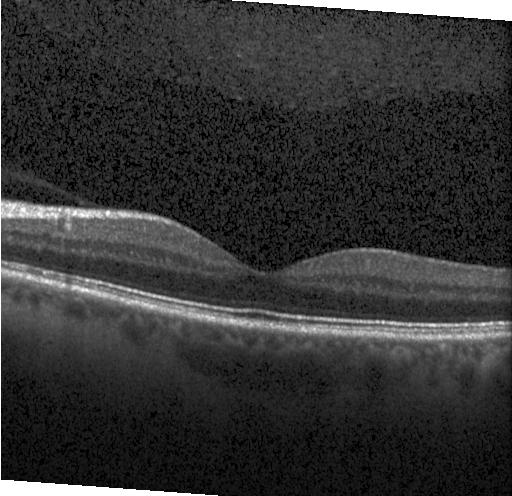 Retinal OCT cross-section. Macular scan. Heidelberg Spectralis. Spectral-domain OCT. Assessment: neither CNV, DME, nor drusen.